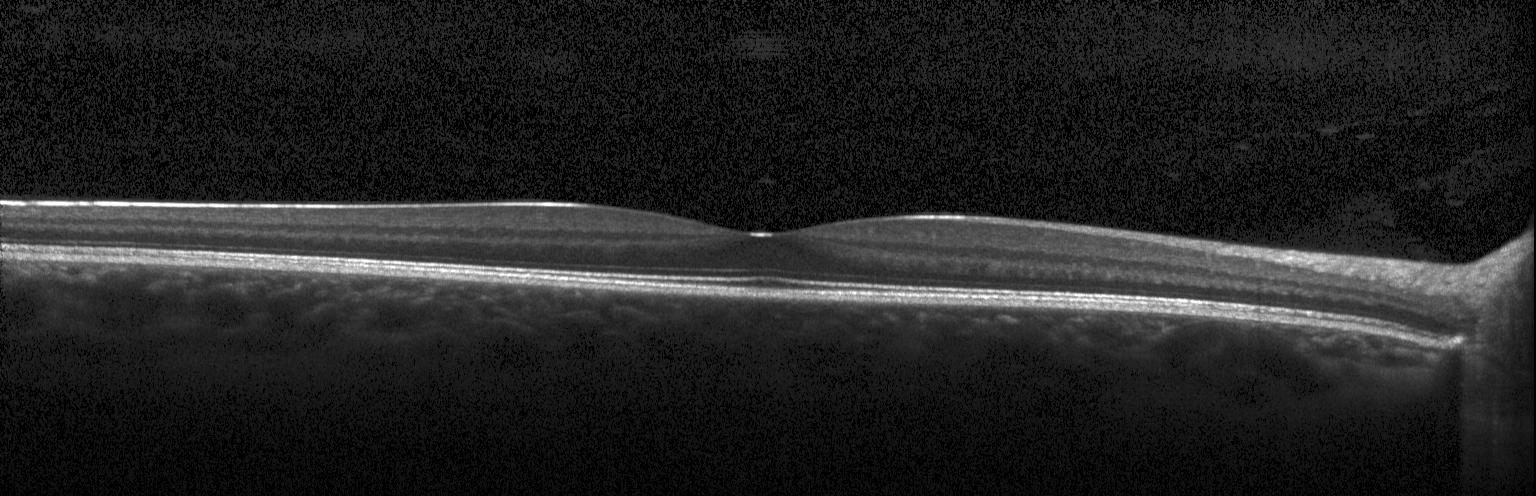 Retinal OCT cross-section. Impression: no choroidal neovascularization, no diabetic macular edema, and no drusen.